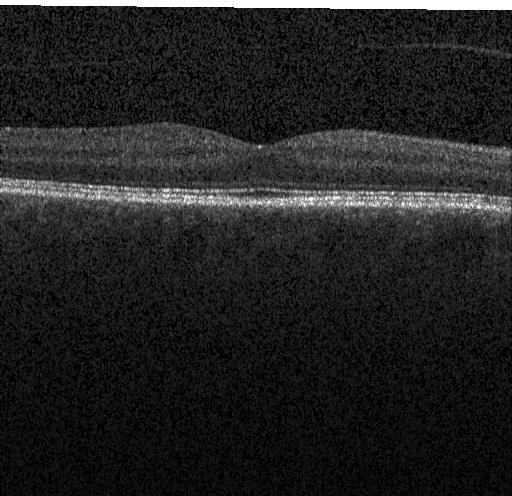 OCT finding: neither CNV, DME, nor drusen.